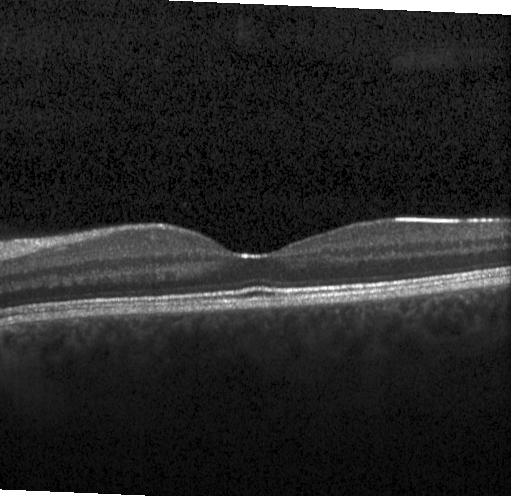 Retinal OCT cross-section.
Finding: no CNV, DME, or drusen.